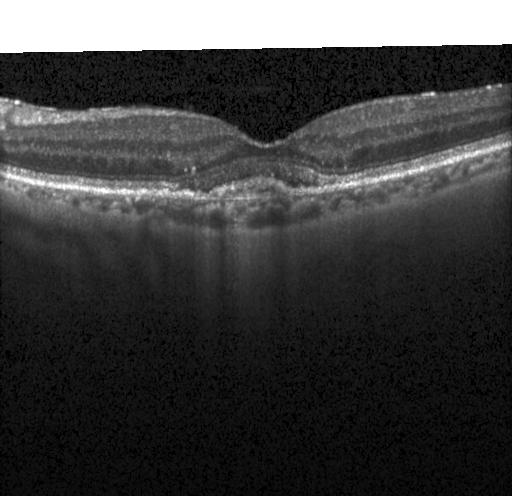
Macular scan · spectral-domain OCT · Heidelberg Spectralis · optical coherence tomography scan — Finding: a choroidal neovascular membrane.